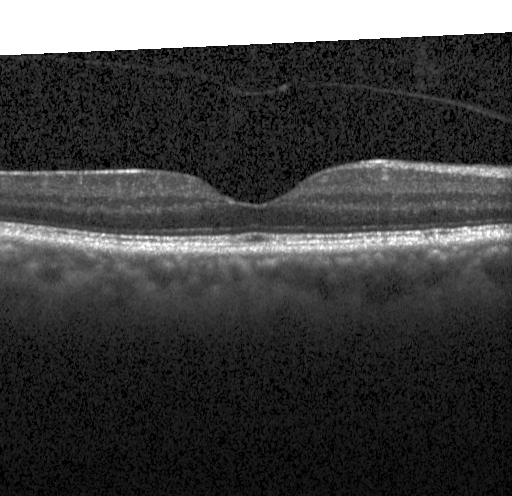
Retinal OCT cross-section showing neither choroidal neovascularization, diabetic macular edema, nor drusen.